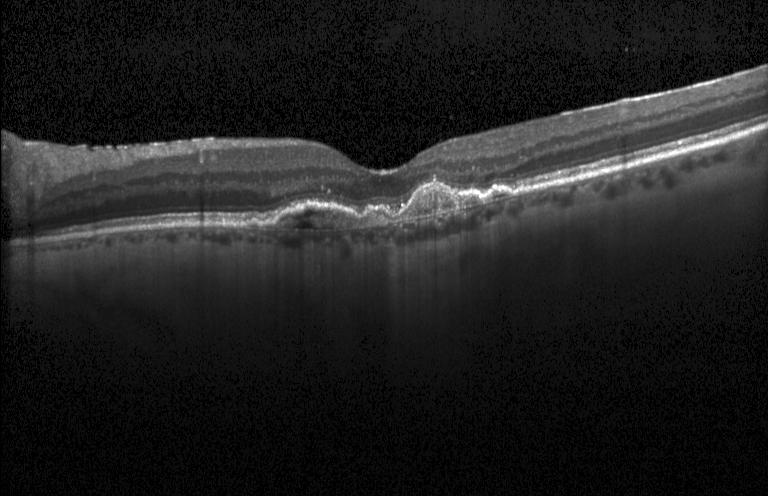 OCT line scan · instrument: Heidelberg Spectralis · fovea-centered. Diagnosis: choroidal neovascularization.